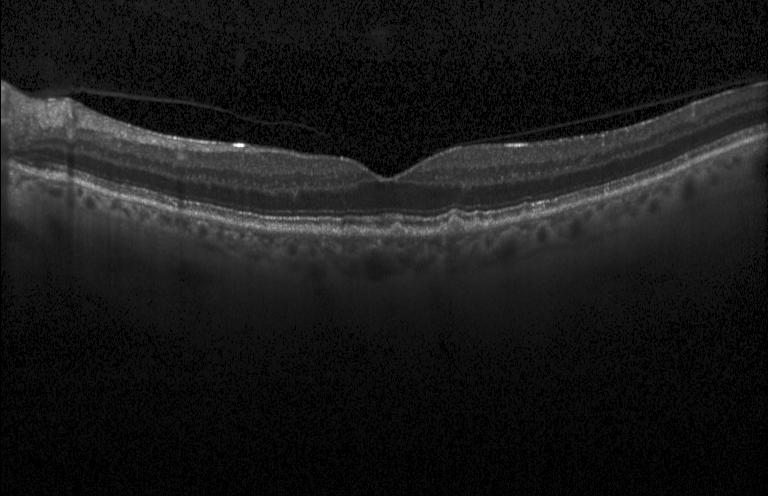

Heidelberg Spectralis; SD-OCT; optical coherence tomography B-scan.
Assessment: multiple drusen.